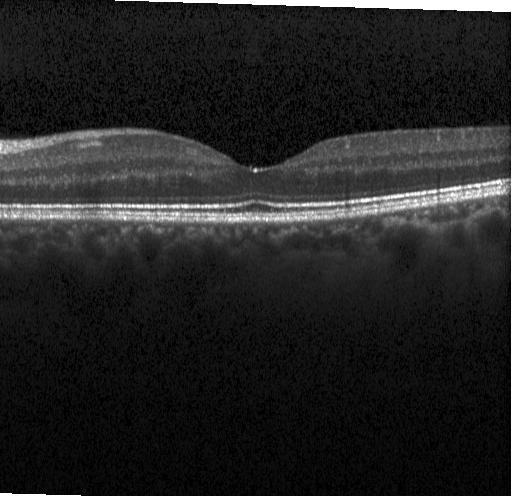 Retinal OCT B-scan · acquired on a Heidelberg Spectralis. Impression: no CNV, DME, or drusen.